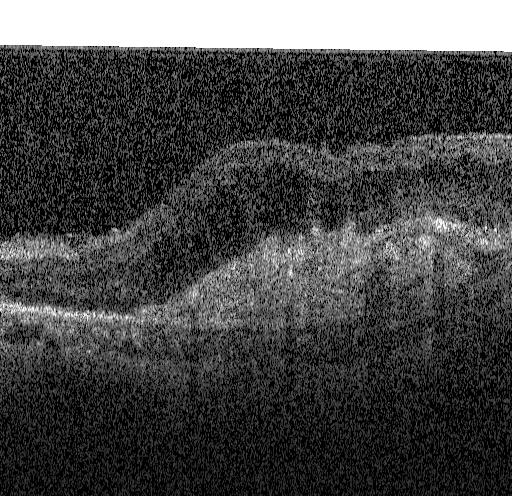
Impression: choroidal neovascularization (CNV).